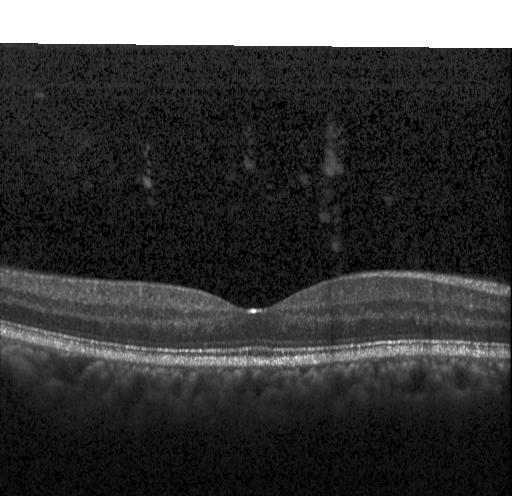 Retinal OCT B-scan, centered on the fovea
OCT finding: no choroidal neovascularization, no diabetic macular edema, and no drusen.